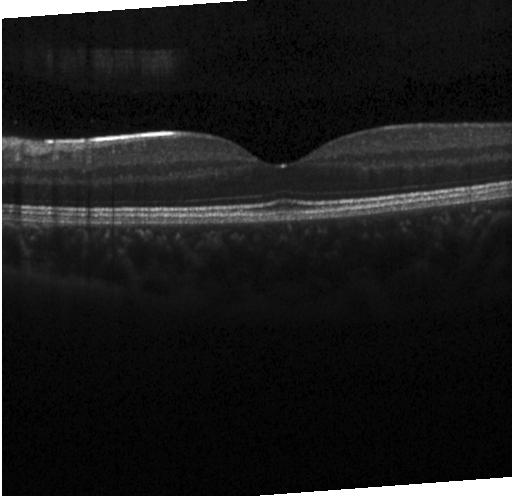 Dx: no CNV, DME, or drusen.